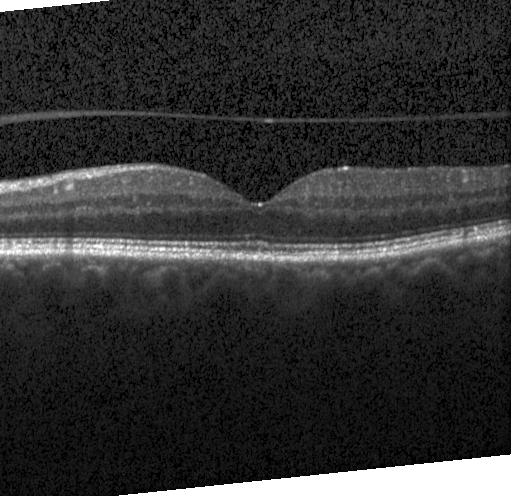

Acquired on a Heidelberg Spectralis. Fovea-centered. Spectral-domain optical coherence tomography. Retinal OCT B-scan
Finding: no CNV, DME, or drusen.